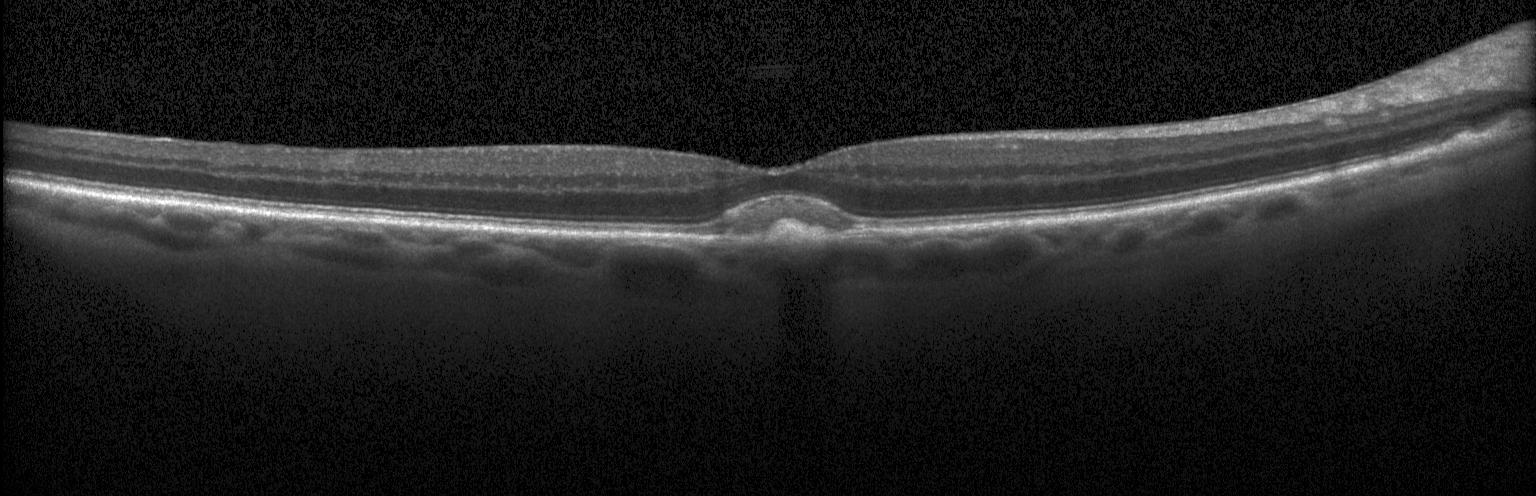

OCT B-scan. Impression: choroidal neovascularization (CNV).